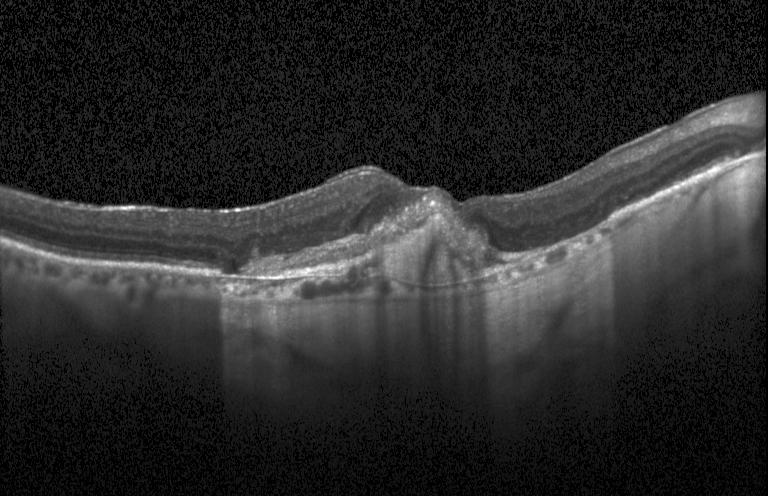

Impression: CNV.